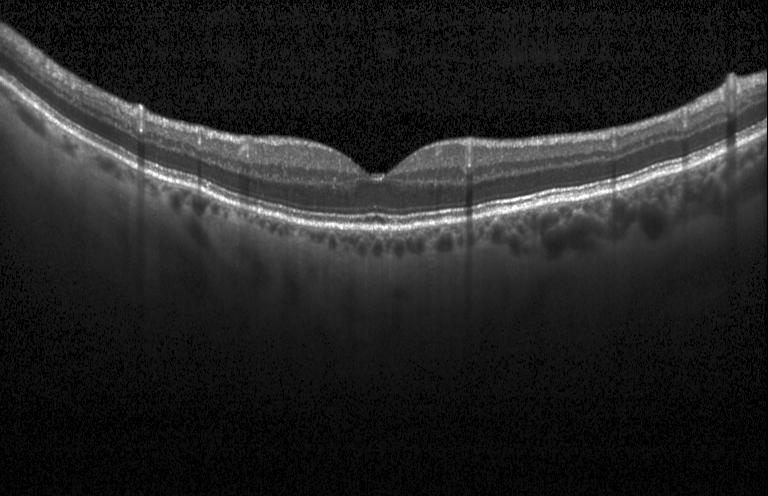

Finding: no CNV, DME, or drusen.